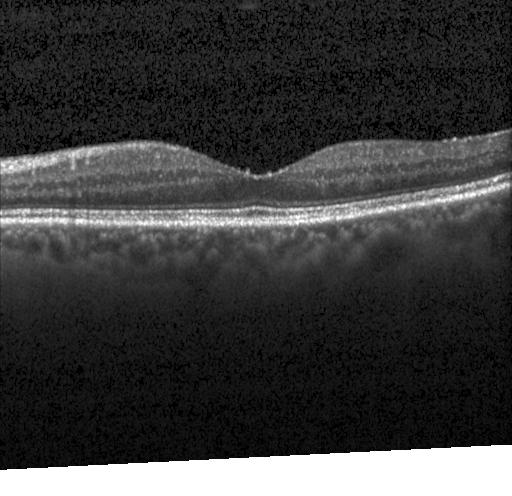 Dx: no choroidal neovascularization, no diabetic macular edema, and no drusen.